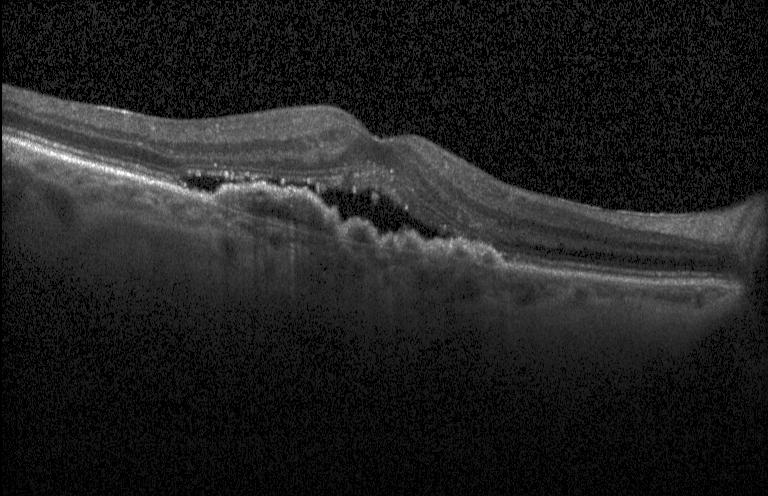
Macular OCT demonstrating CNV.